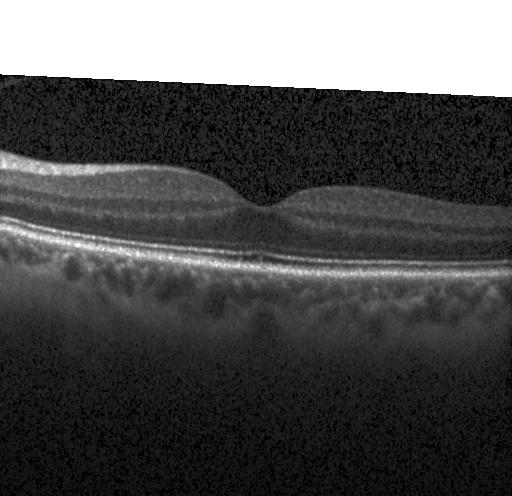 Retinal OCT cross-section. Impression: neither choroidal neovascularization, diabetic macular edema, nor drusen.